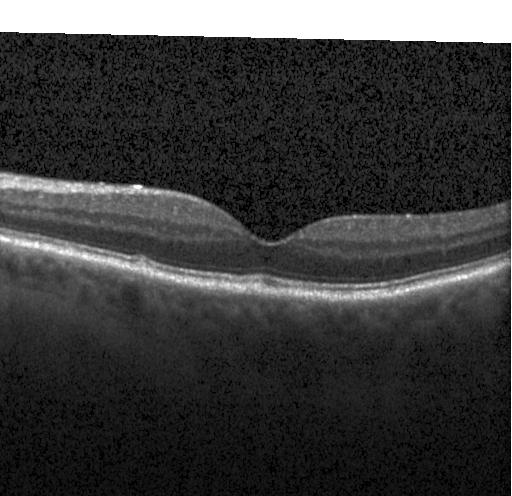 Heidelberg Spectralis · through the macula · spectral-domain optical coherence tomography · OCT line scan — Assessment: sub-RPE drusenoid deposits.